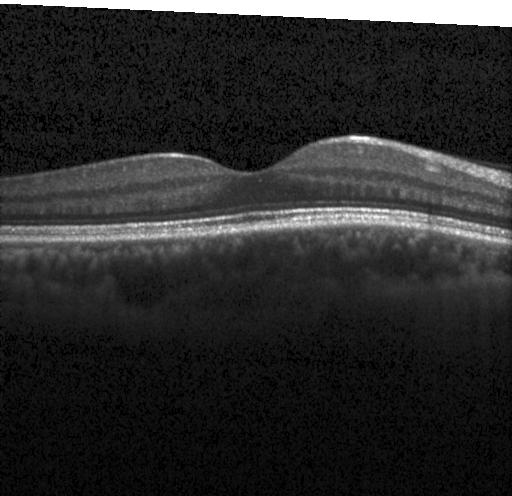

Acquired on a Heidelberg Spectralis · spectral-domain optical coherence tomography · optical coherence tomography B-scan. Diagnosis: no choroidal neovascularization, diabetic macular edema, or drusen.